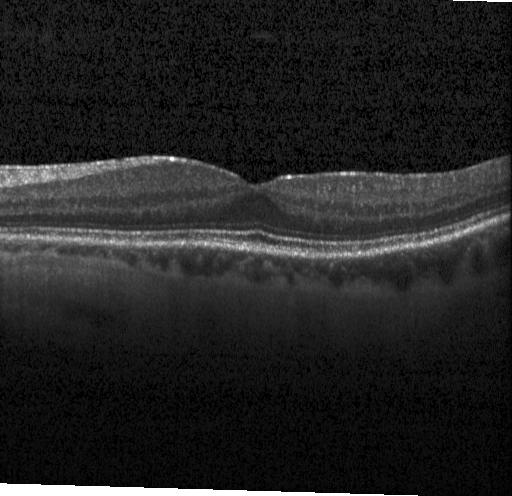

Impression: no choroidal neovascularization, no diabetic macular edema, and no drusen.